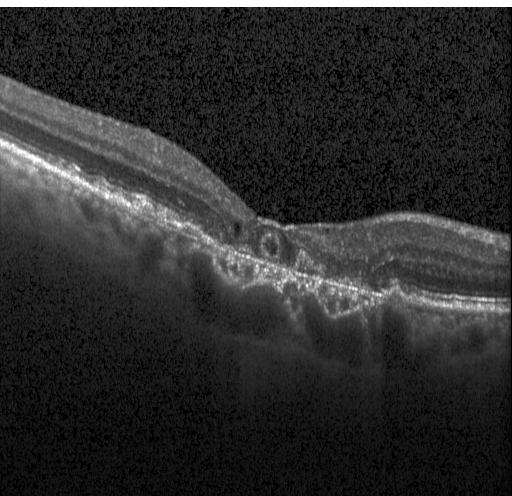
OCT finding: a choroidal neovascular membrane.